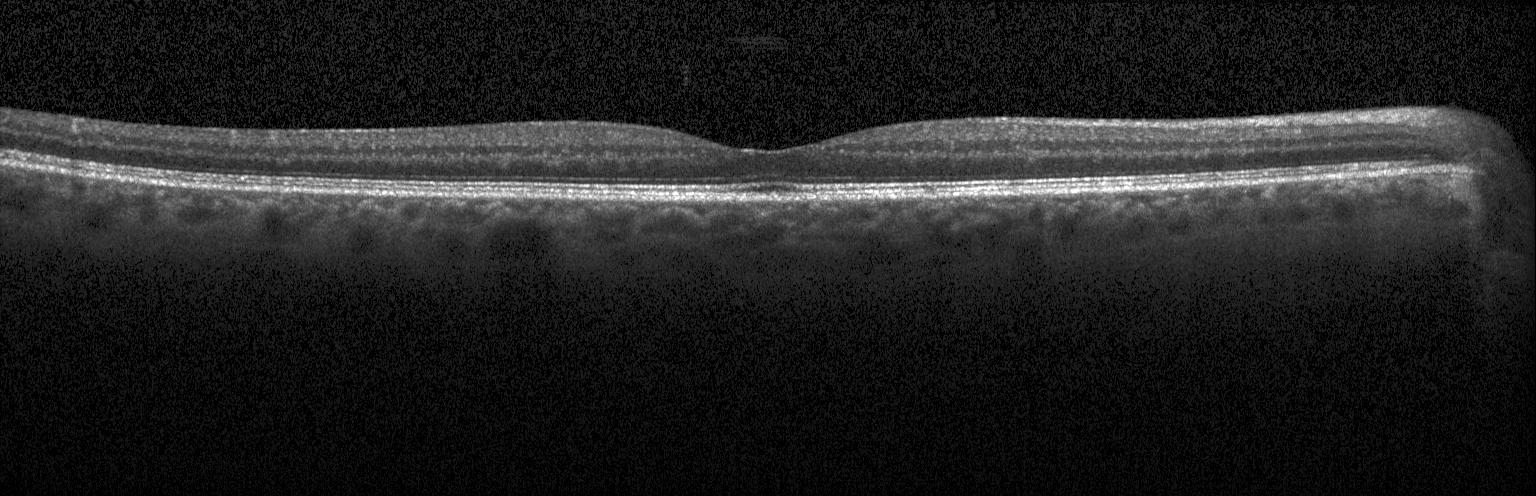 Through the macula; retinal OCT cross-section; Heidelberg Spectralis
Assessment: no CNV, no DME, and no drusen.